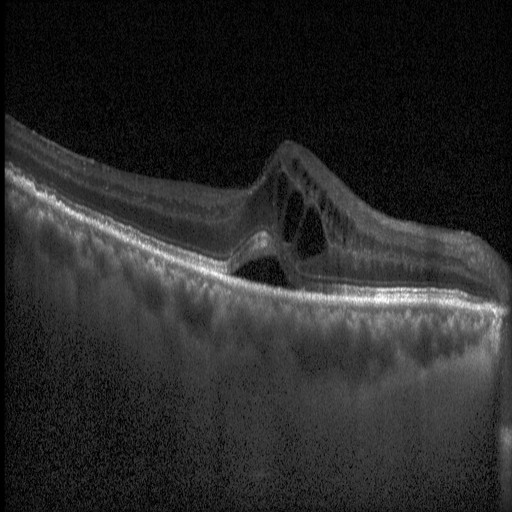

Finding: DME.